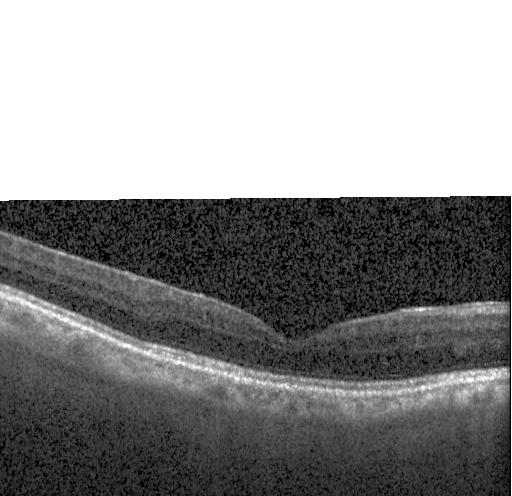

Optical coherence tomography scan; spectral-domain OCT
Neither CNV, DME, nor drusen.